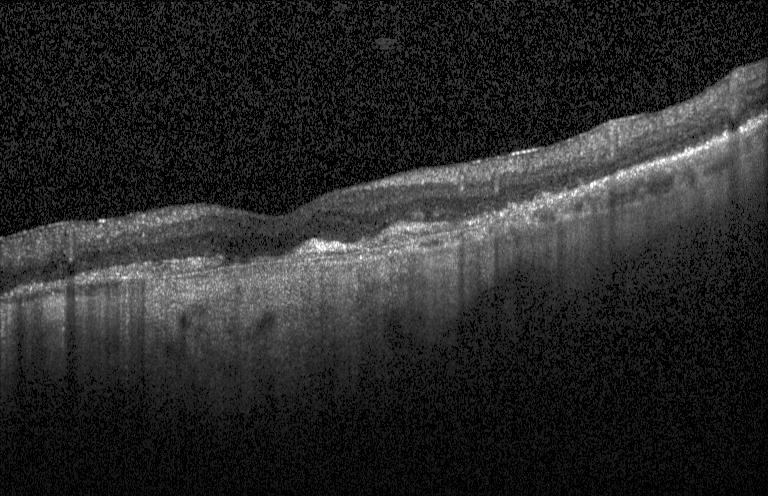
Spectral-domain OCT, through the macula, optical coherence tomography B-scan.
This B-scan demonstrates a choroidal neovascular membrane.